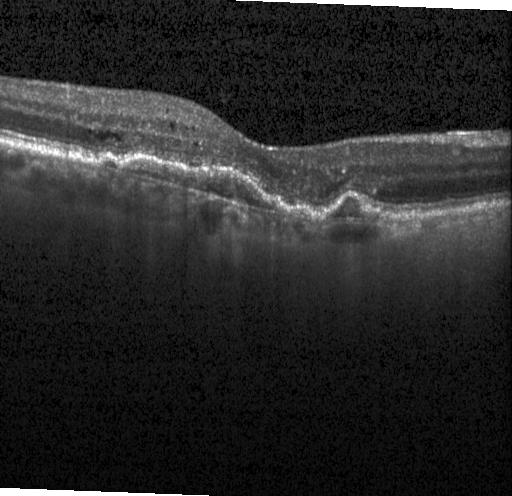
SD-OCT · OCT B-scan · through the macula — The scan shows choroidal neovascularization.